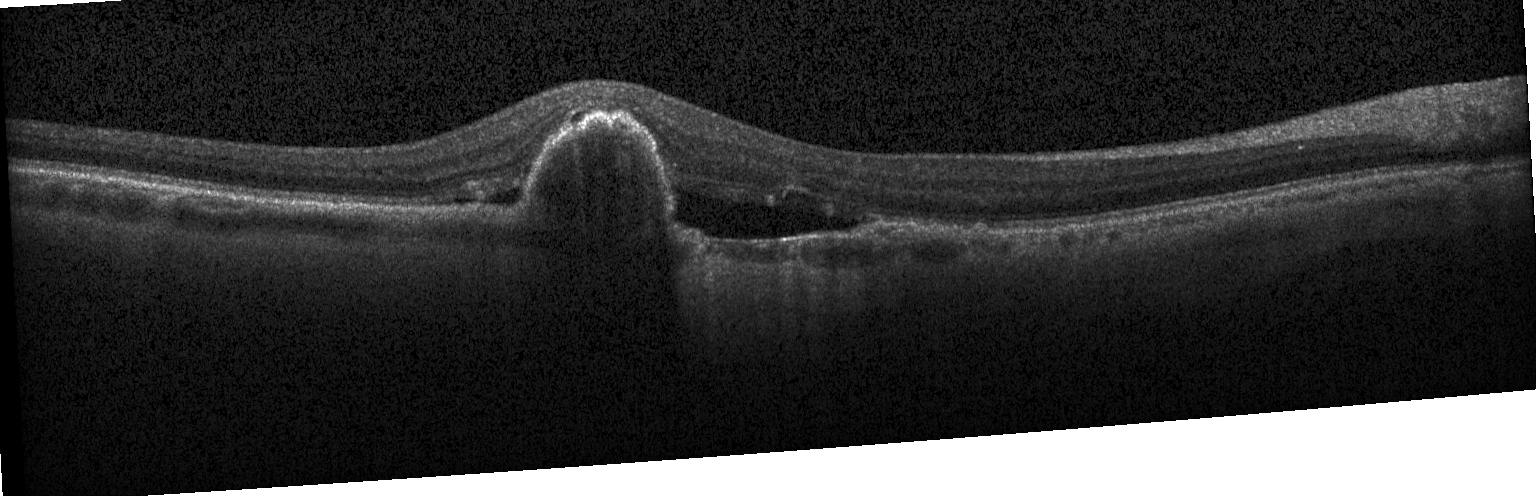
Through the macula · SD-OCT · optical coherence tomography B-scan — This B-scan demonstrates CNV.